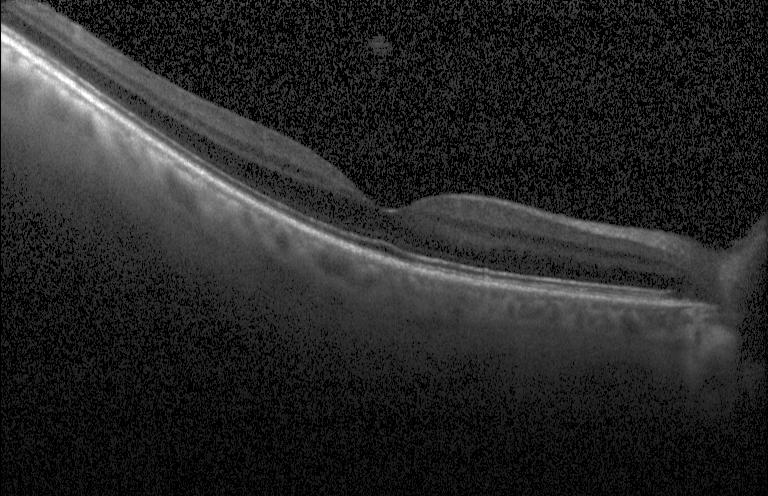

OCT B-scan.
The scan shows neither choroidal neovascularization, diabetic macular edema, nor drusen.